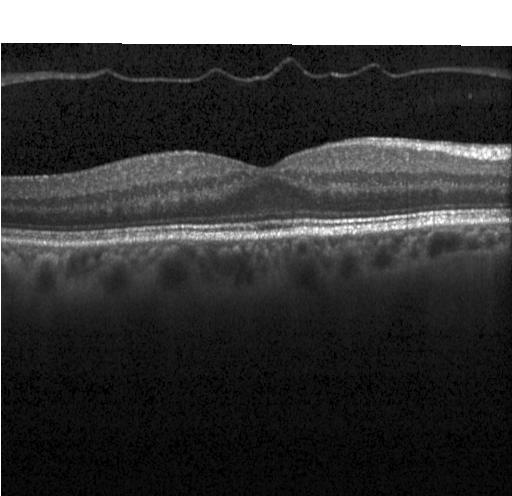
Spectral-domain optical coherence tomography · retinal OCT B-scan. Finding: no choroidal neovascularization, diabetic macular edema, or drusen.